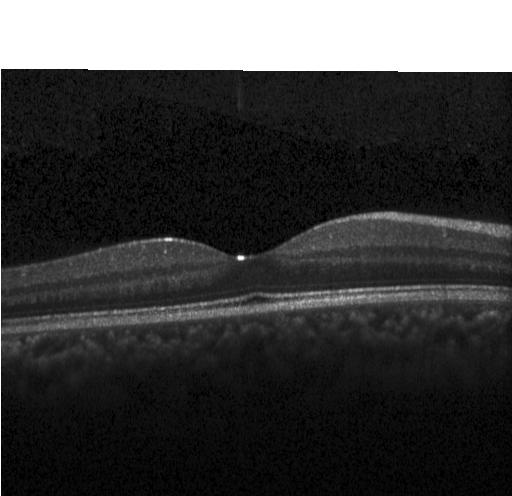
Retinal OCT cross-section, spectral-domain OCT. Dx: no choroidal neovascularization, no diabetic macular edema, and no drusen.